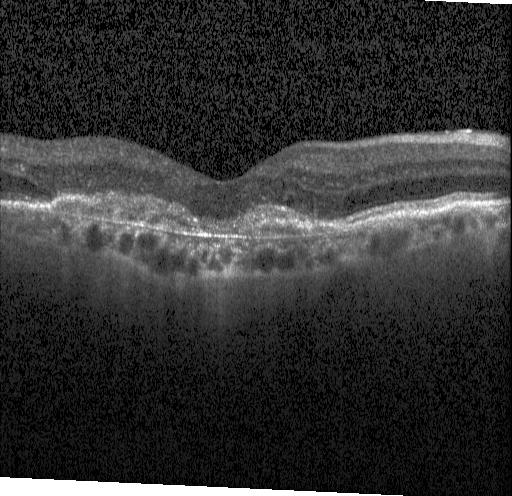
Retinal OCT cross-section showing a choroidal neovascular membrane.